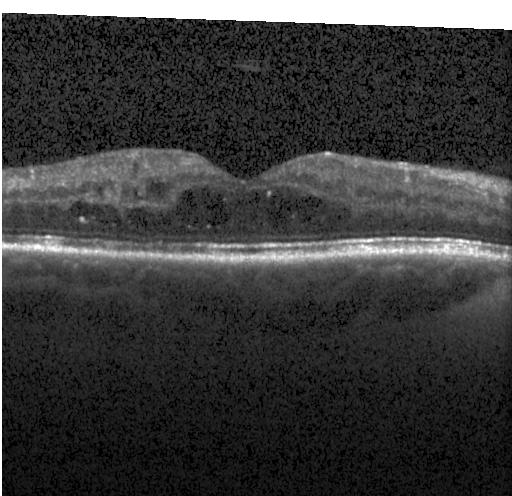 Heidelberg Spectralis, centered on the fovea, spectral-domain OCT, retinal OCT cross-section — Assessment: diabetic macular edema.